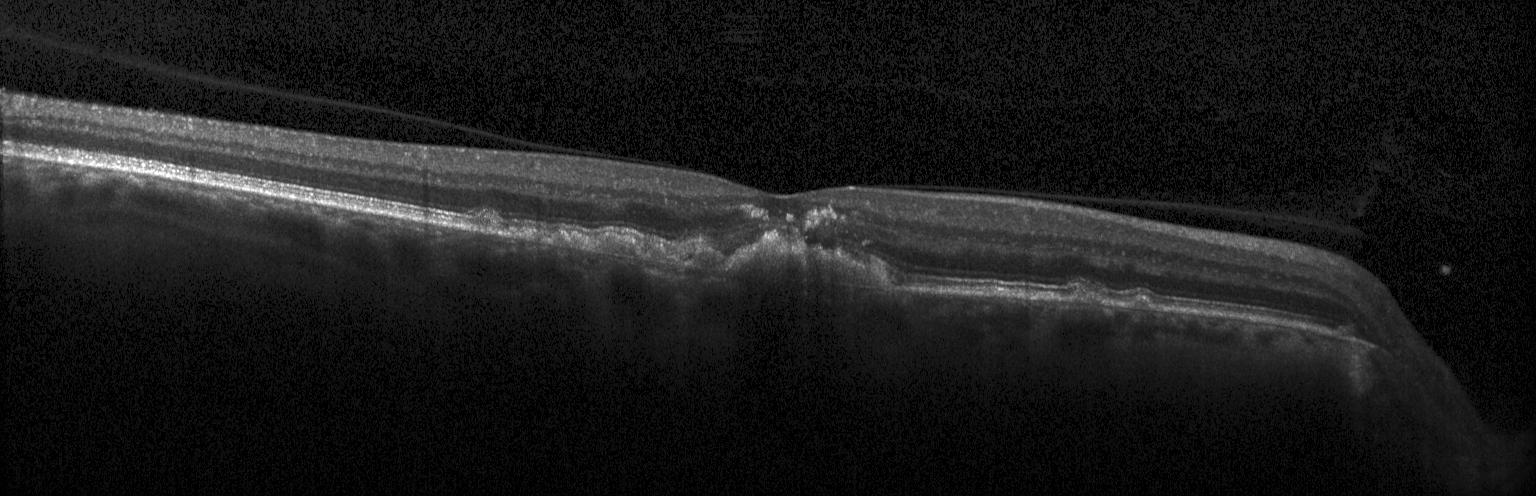

Optical coherence tomography B-scan. Dx: CNV.